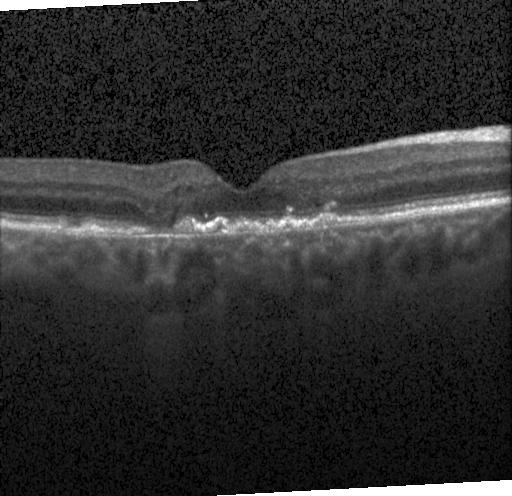 Heidelberg Spectralis, retinal OCT B-scan, spectral-domain optical coherence tomography, through the macula.
This B-scan demonstrates CNV.